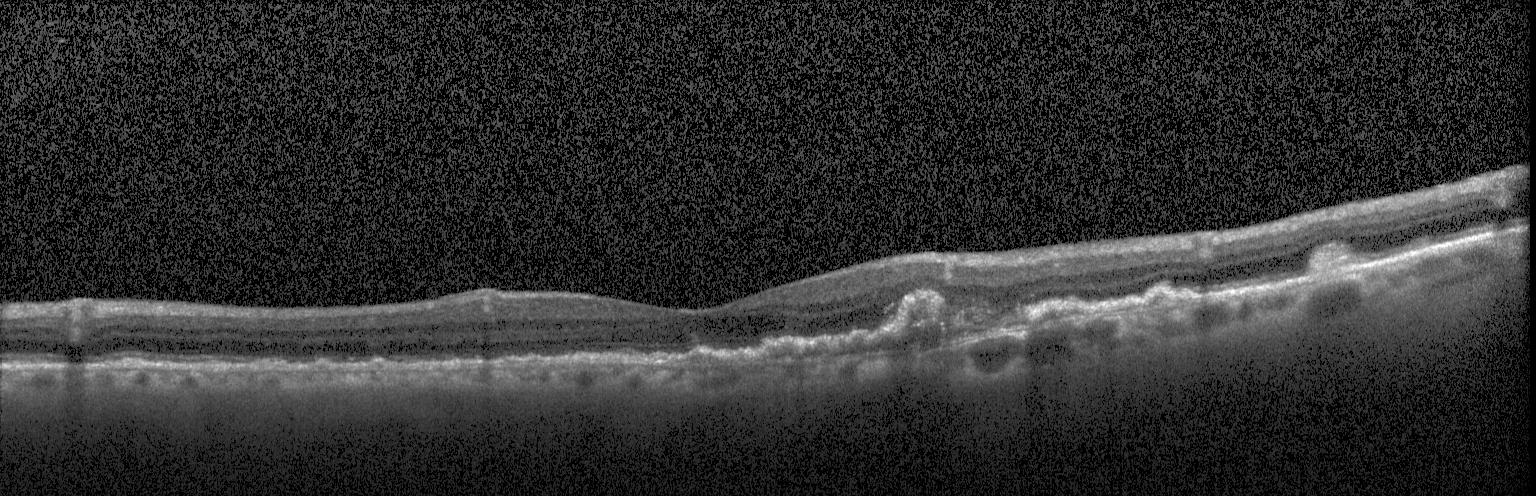
OCT B-scan showing a choroidal neovascular membrane.